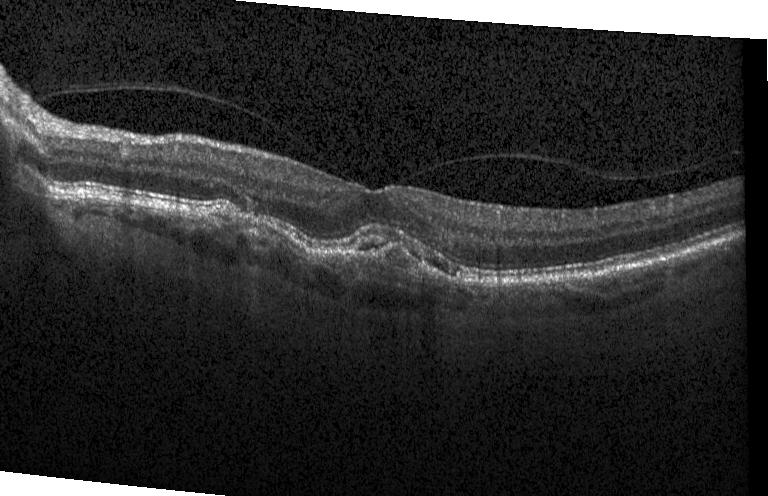
Retinal OCT cross-section, acquired on a Heidelberg Spectralis
Diagnosis: CNV.